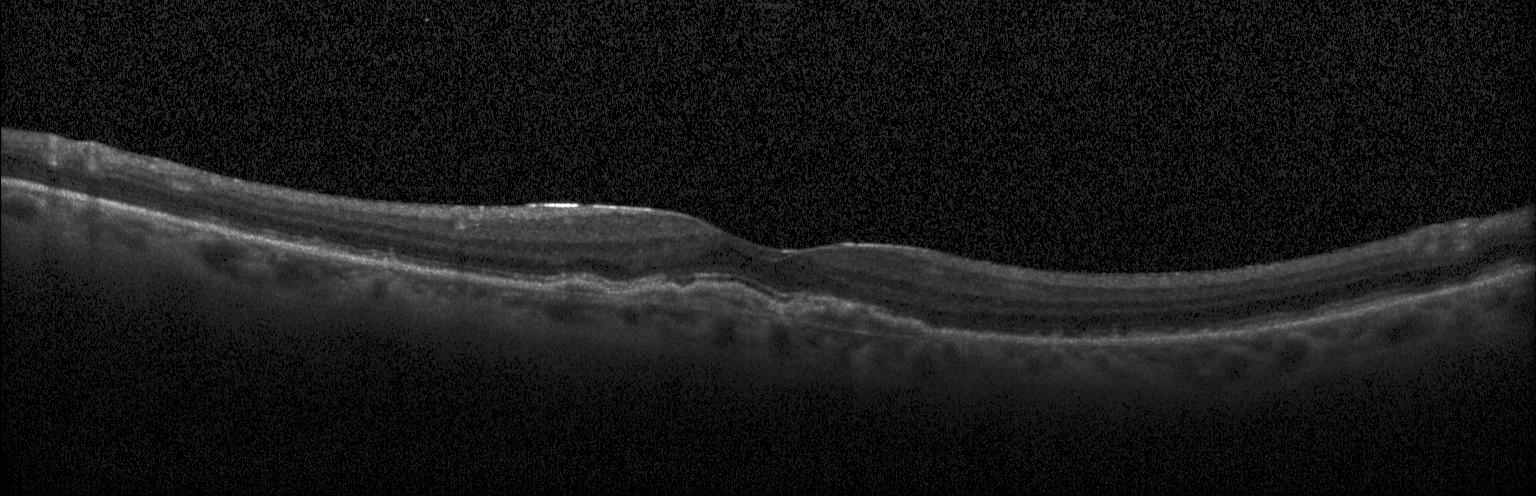

Retinal OCT cross-section — Finding: choroidal neovascularization.